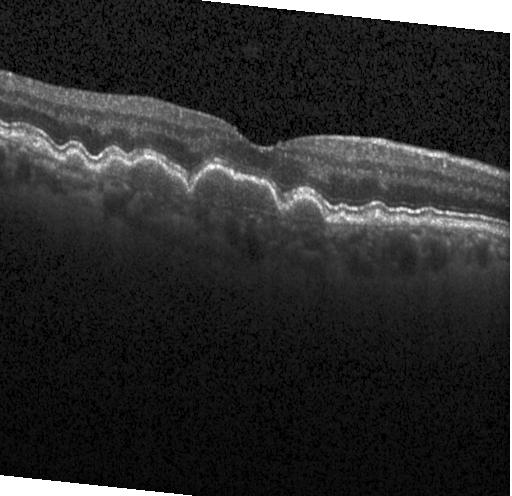 Optical coherence tomography scan; spectral-domain optical coherence tomography. This B-scan demonstrates sub-RPE drusenoid deposits.